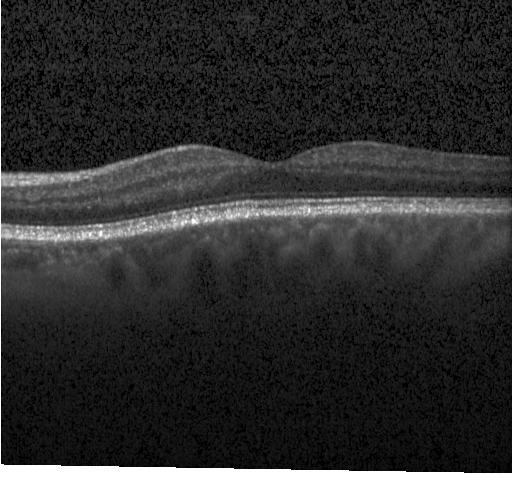

SD-OCT. Fovea-centered. Heidelberg Spectralis OCT system. Retinal OCT B-scan. Assessment: no choroidal neovascularization, diabetic macular edema, or drusen.